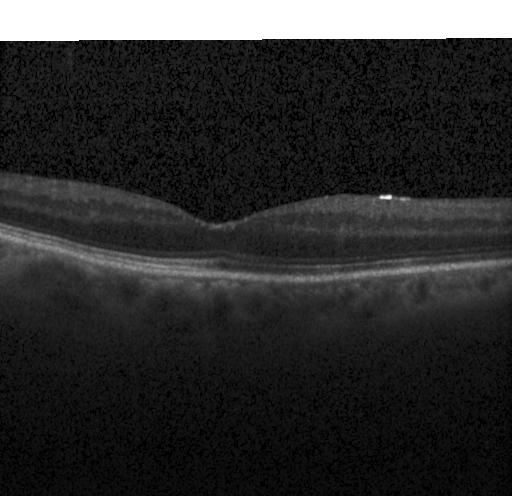

Retinal OCT B-scan. Diagnosis: neither choroidal neovascularization, diabetic macular edema, nor drusen.